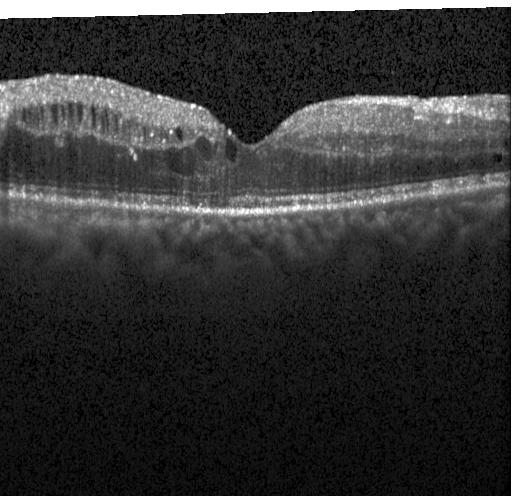

Impression: diabetic macular edema.